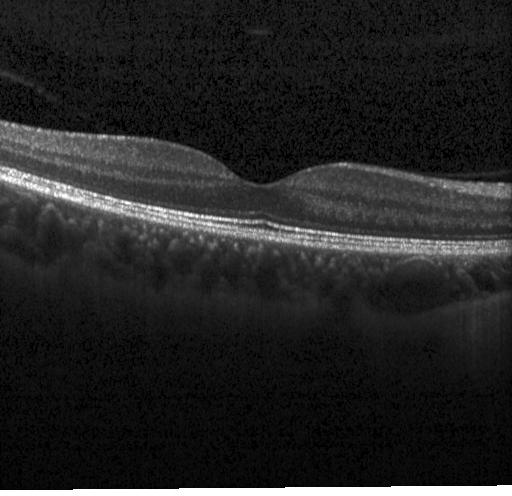
Heidelberg Spectralis OCT system. Through the macula. Optical coherence tomography B-scan — Dx: no choroidal neovascularization, no diabetic macular edema, and no drusen.